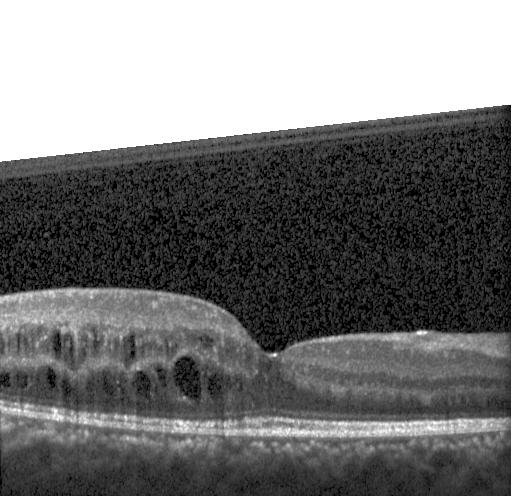

Spectral-domain OCT B-scan: diabetic macular edema.